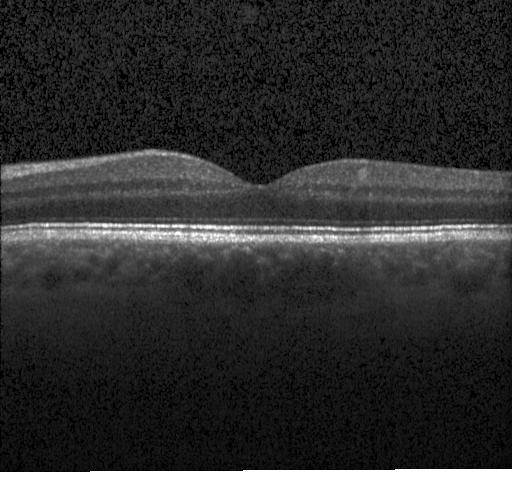
Optical coherence tomography scan
Impression: neither choroidal neovascularization, diabetic macular edema, nor drusen.